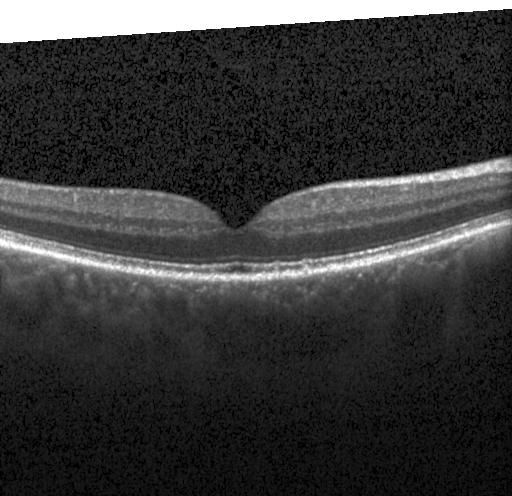
Retinal OCT cross-section; instrument: Heidelberg Spectralis.
The scan shows no CNV, DME, or drusen.